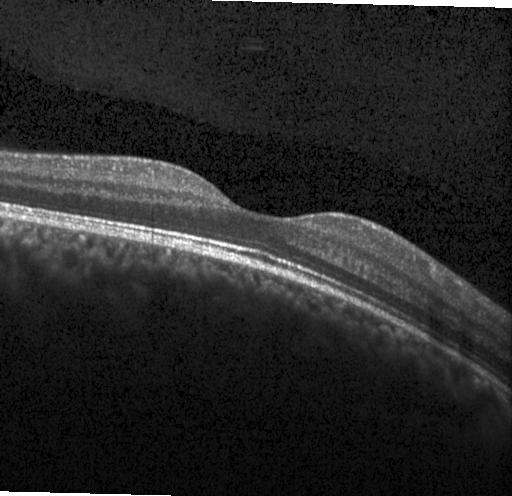

Heidelberg Spectralis · fovea-centered · OCT line scan. OCT finding: neither choroidal neovascularization, diabetic macular edema, nor drusen.